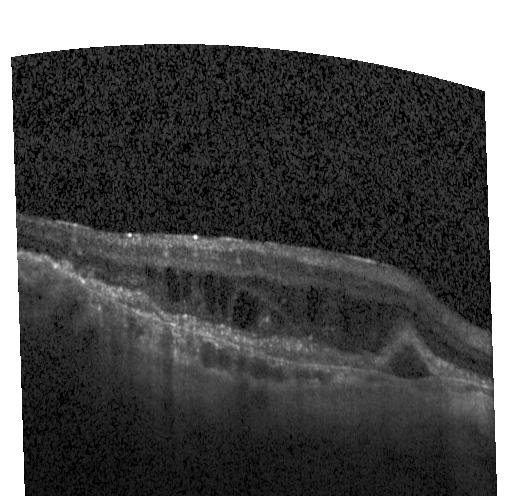
Macular OCT: choroidal neovascularization (CNV).